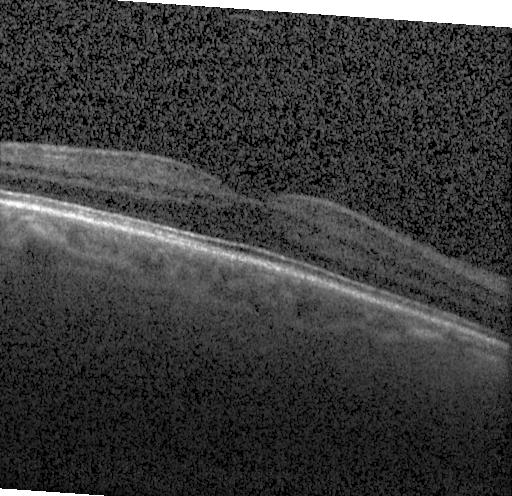 Spectral-domain OCT, OCT line scan. Finding: no CNV, no DME, and no drusen.